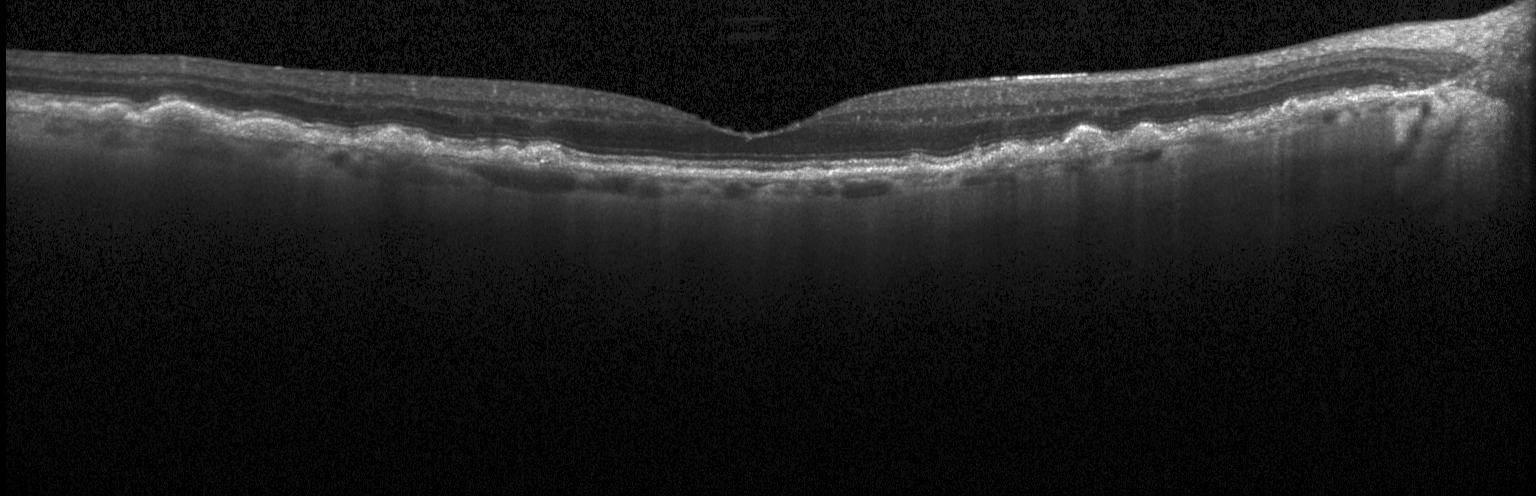 Drusen.